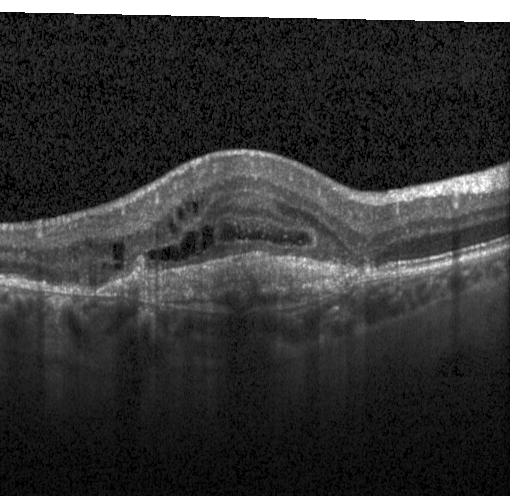
This B-scan demonstrates a choroidal neovascular membrane.